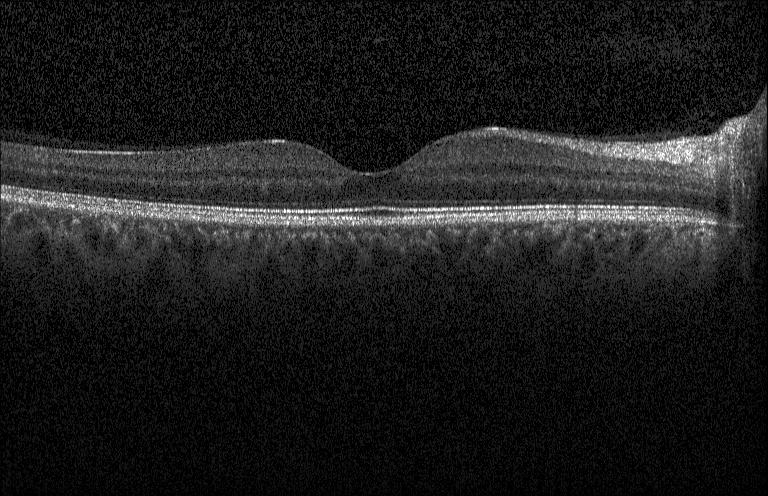 OCT line scan; Heidelberg Spectralis OCT system
Impression: no evidence of choroidal neovascularization, diabetic macular edema, or drusen.